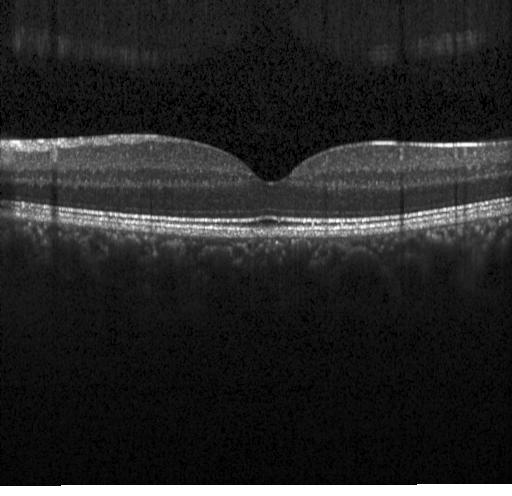 SD-OCT. Heidelberg Spectralis OCT system. Retinal OCT B-scan.
OCT finding: no CNV, DME, or drusen.